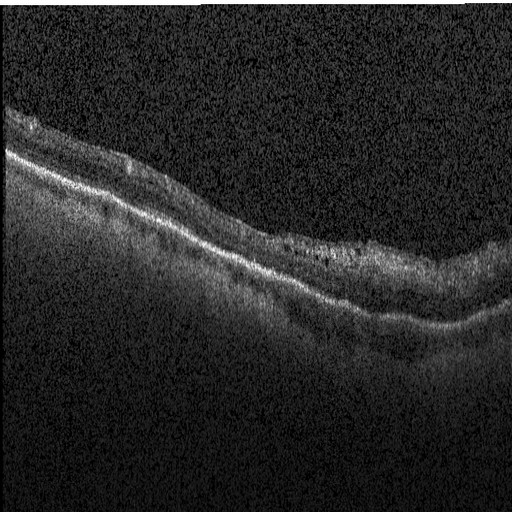
Impression: diabetic macular edema.